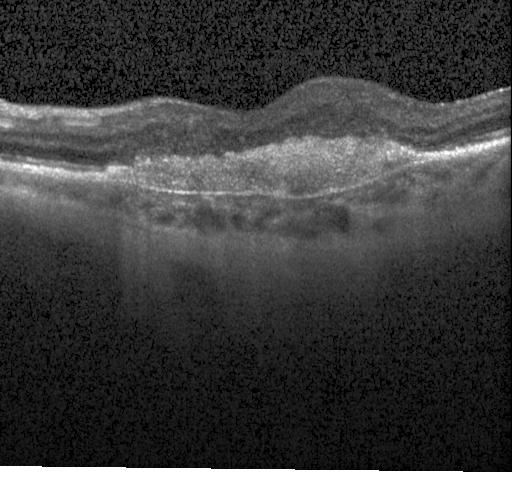 Acquired on a Heidelberg Spectralis. Spectral-domain optical coherence tomography. Retinal OCT B-scan. Dx: choroidal neovascularization (CNV).